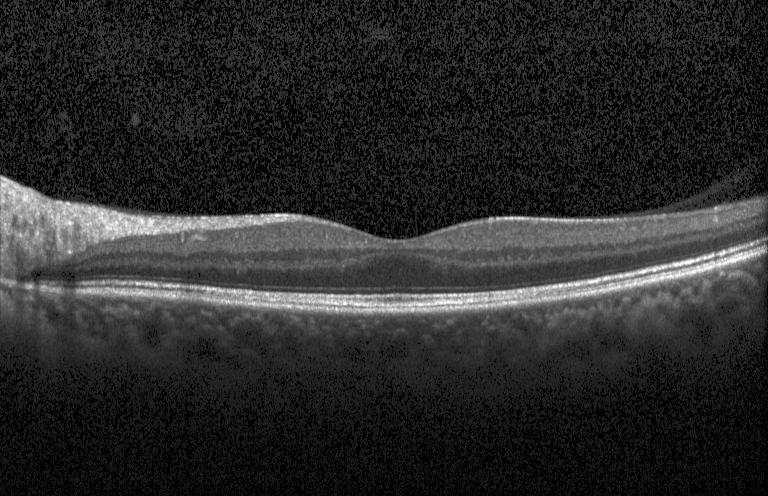
Spectral-domain OCT B-scan: no evidence of choroidal neovascularization, diabetic macular edema, or drusen.